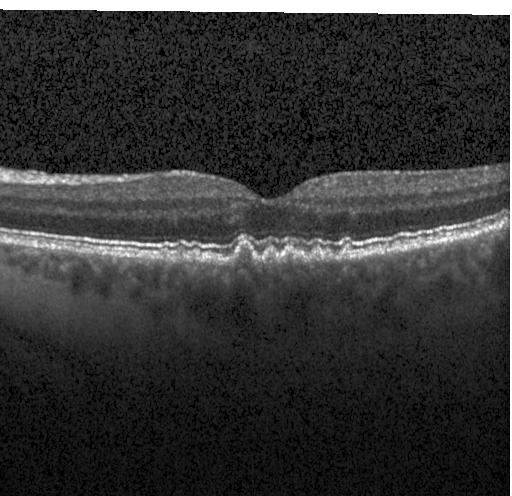

Retinal OCT cross-section showing drusen.